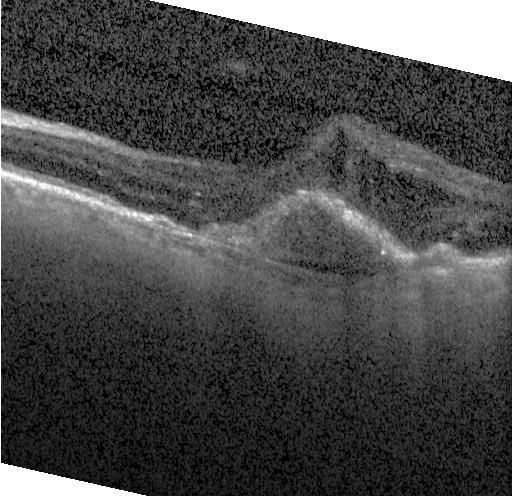
Macular OCT: a choroidal neovascular membrane.